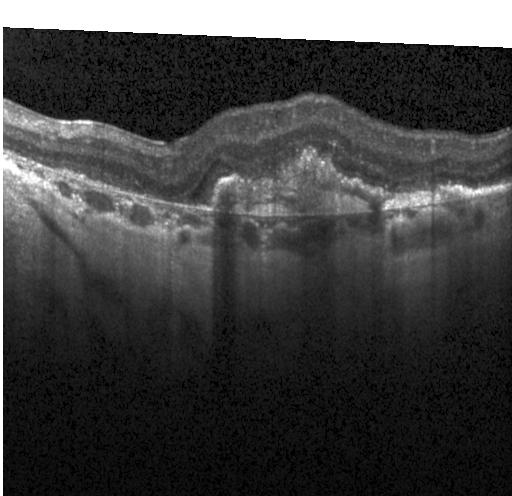 Impression: a choroidal neovascular membrane.